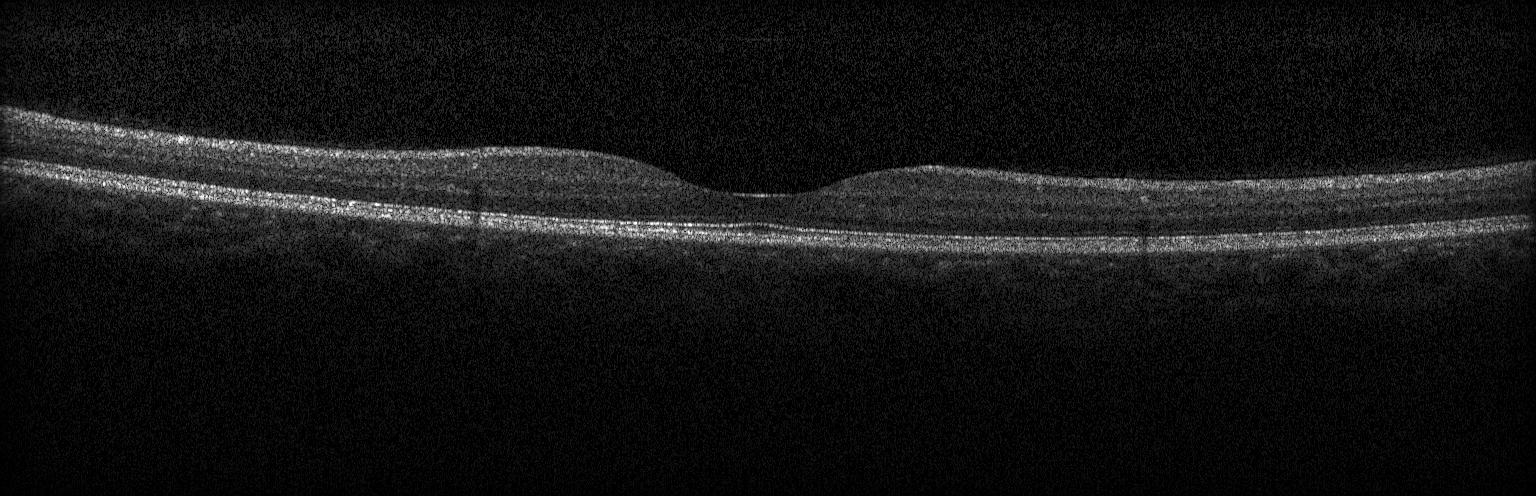
Spectral-domain OCT B-scan: no evidence of CNV, DME, or drusen.